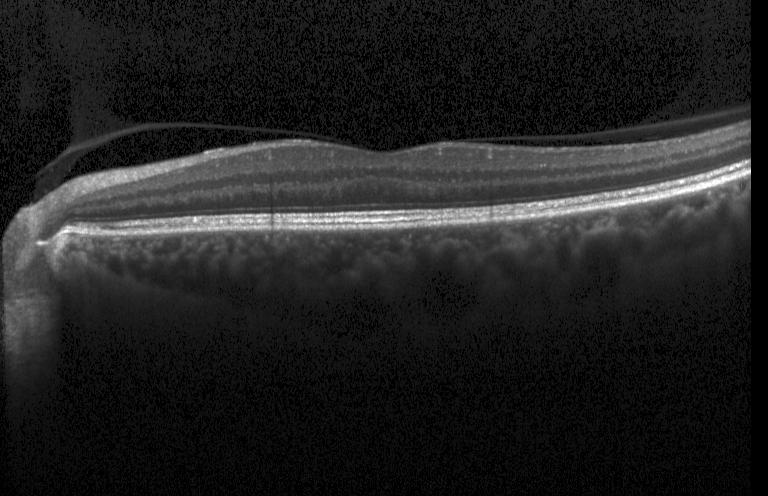

Assessment: no choroidal neovascularization, diabetic macular edema, or drusen.